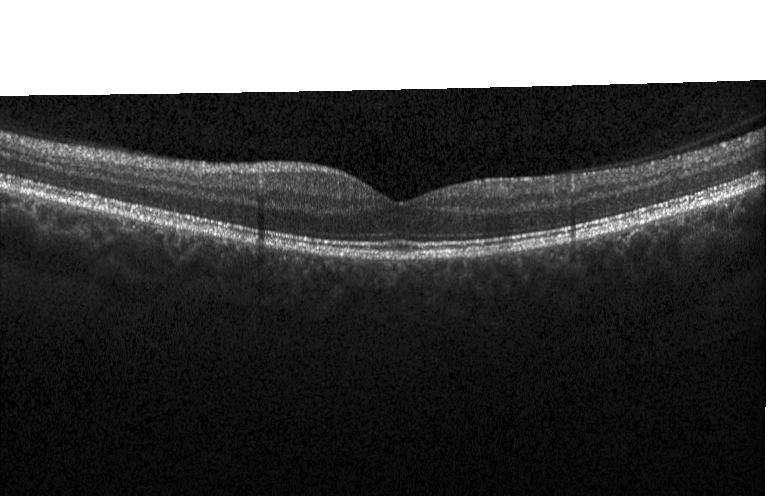

OCT line scan — Diagnosis: no choroidal neovascularization, diabetic macular edema, or drusen.